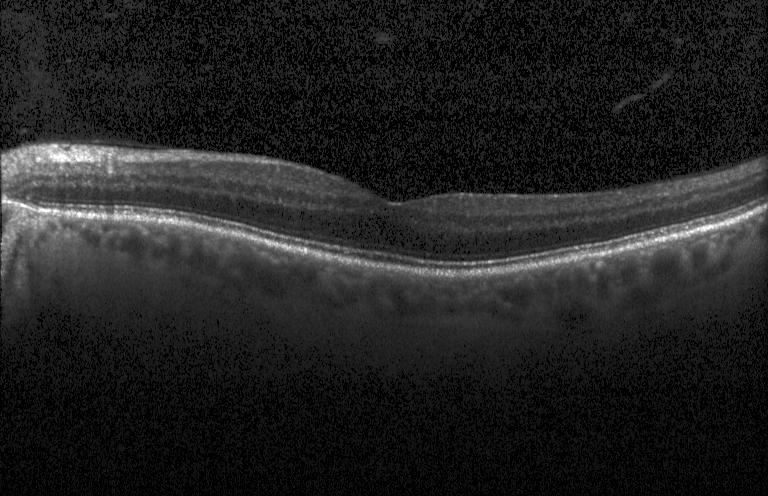
Spectral-domain optical coherence tomography · Heidelberg Spectralis · OCT B-scan — Assessment: no choroidal neovascularization, diabetic macular edema, or drusen.